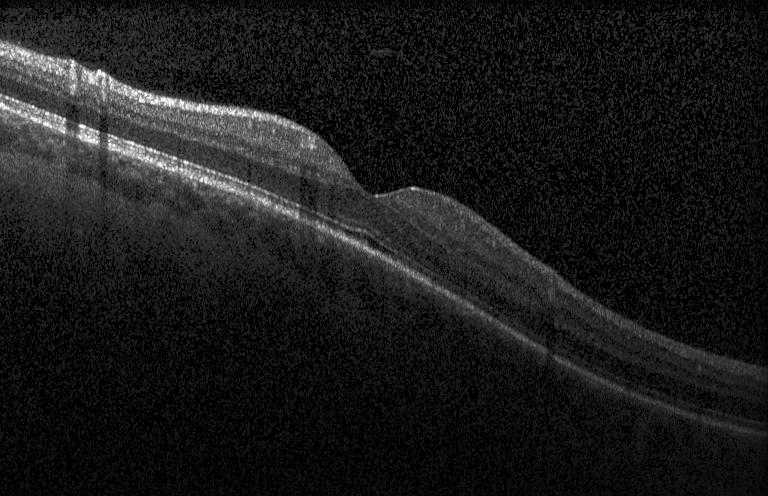
OCT scan showing neither CNV, DME, nor drusen.